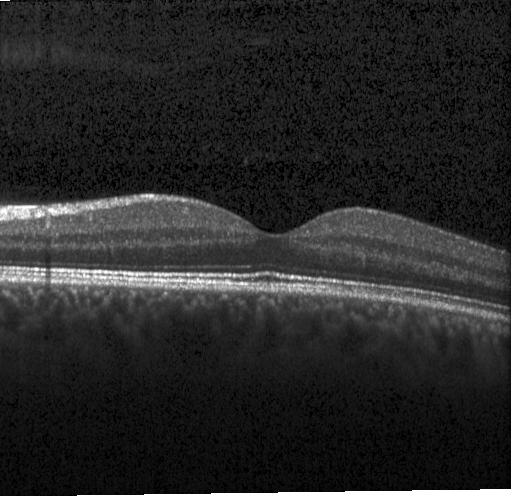
OCT B-scan
Finding: no choroidal neovascularization, no diabetic macular edema, and no drusen.